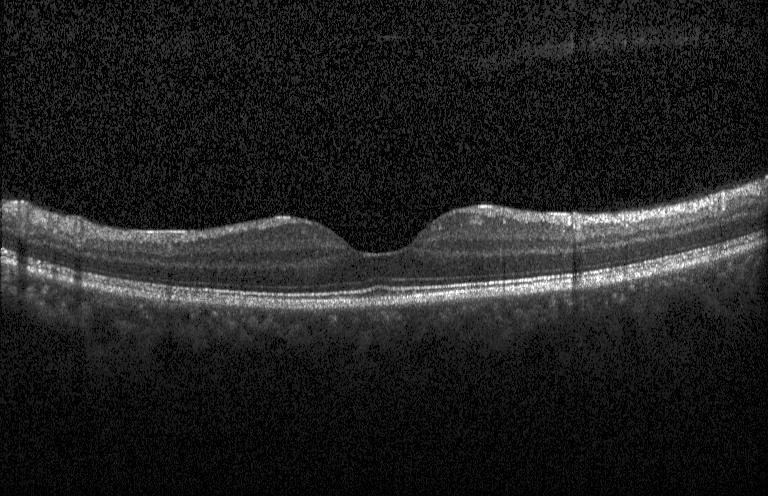 Horizontal scan through the fovea, optical coherence tomography scan.
Finding: no CNV, no DME, and no drusen.